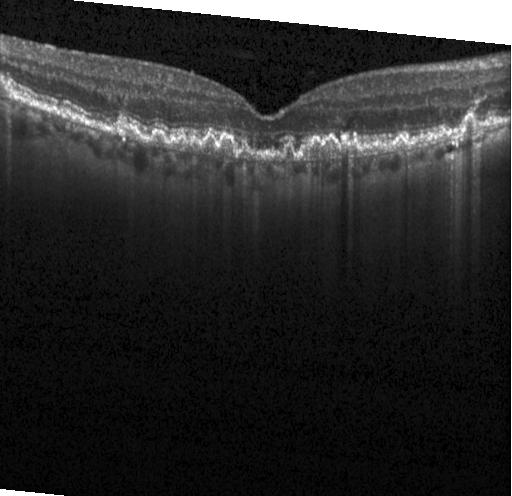
Diagnosis: sub-RPE drusenoid deposits.